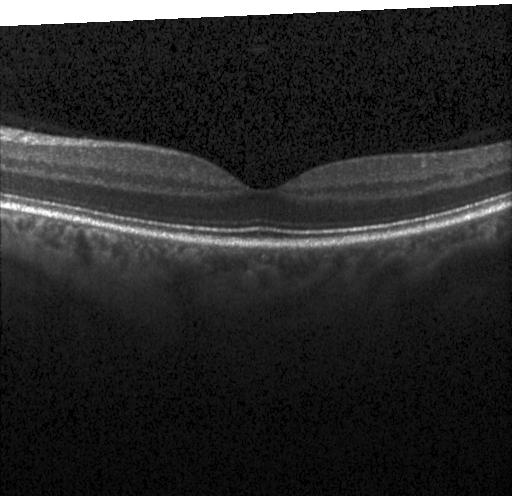 Fovea-centered, retinal OCT B-scan.
Finding: no evidence of choroidal neovascularization, diabetic macular edema, or drusen.